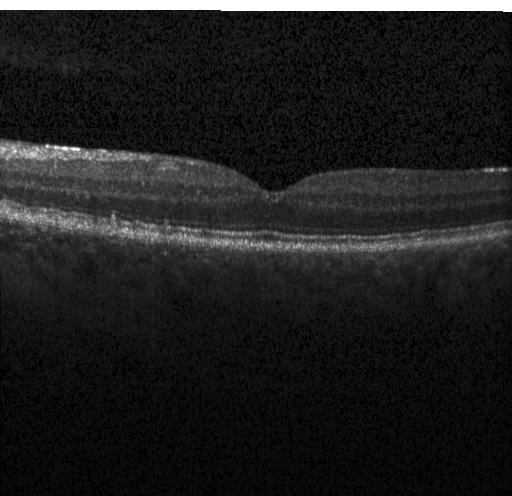

Fovea-centered; instrument: Heidelberg Spectralis; OCT B-scan; SD-OCT.
The scan shows multiple drusen.